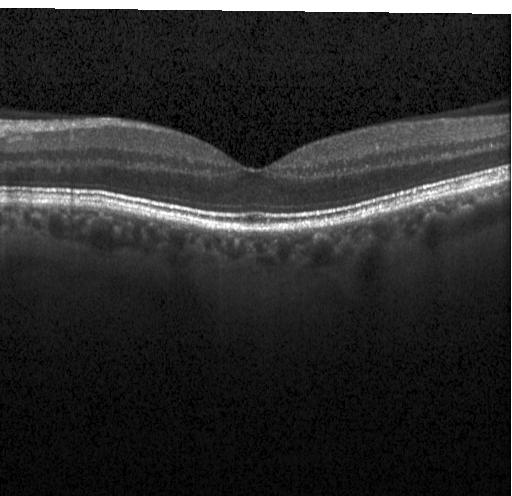 Horizontal scan through the fovea, Heidelberg Spectralis, OCT line scan, spectral-domain optical coherence tomography — Impression: neither CNV, DME, nor drusen.